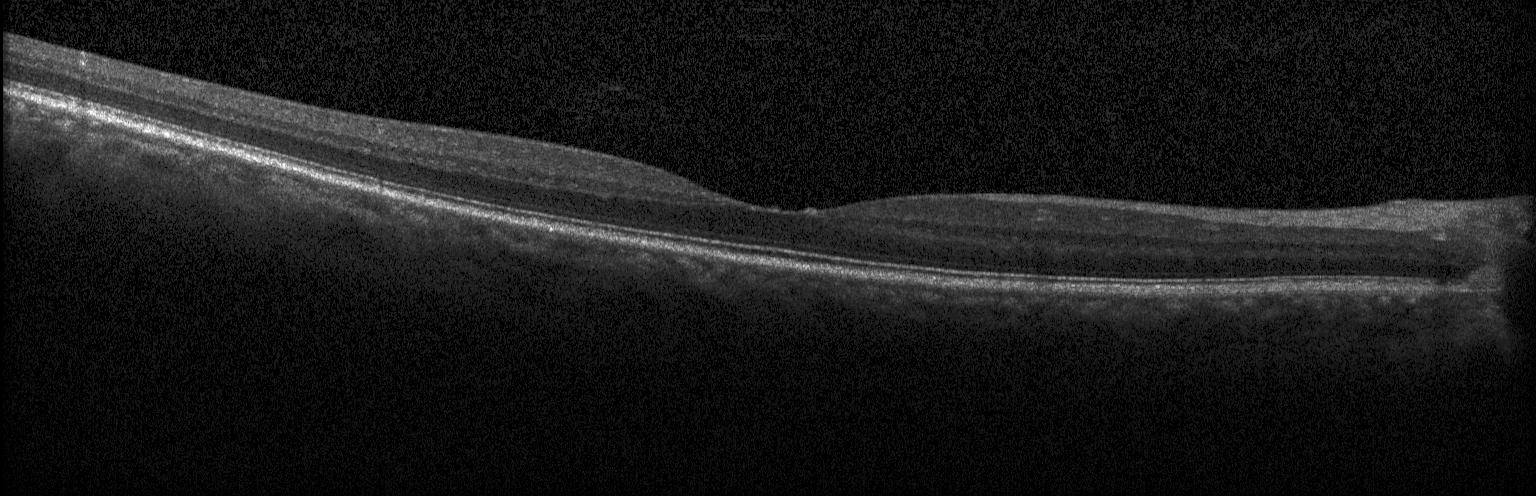
OCT line scan · horizontal scan through the fovea. Diagnosis: no evidence of choroidal neovascularization, diabetic macular edema, or drusen.